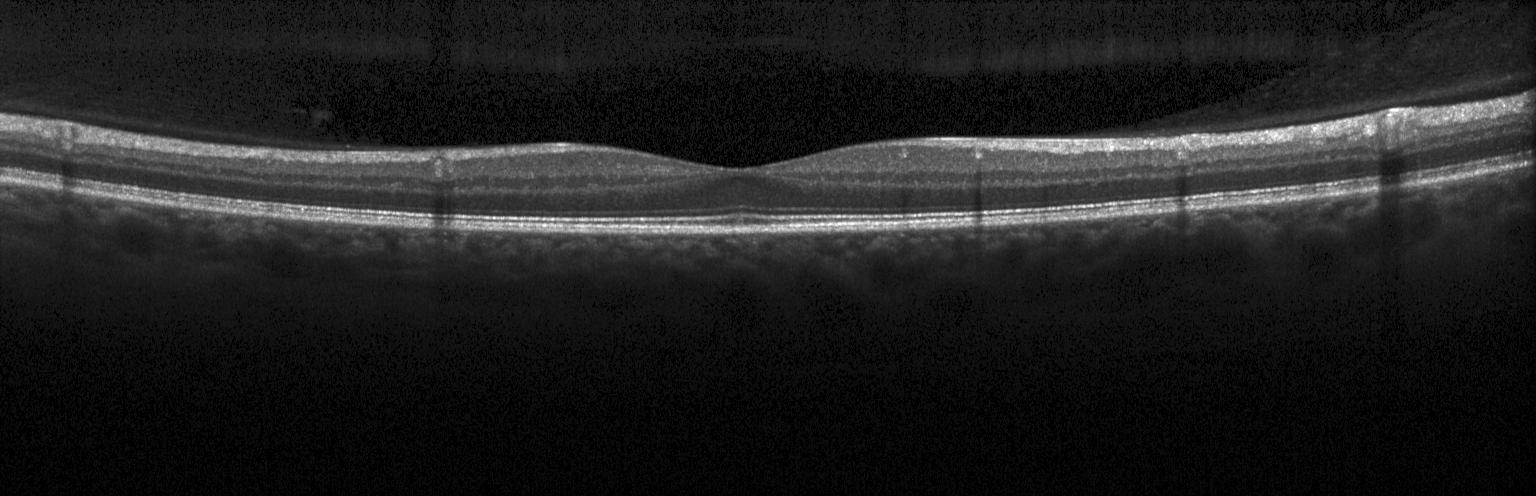
Macular OCT demonstrating no CNV, DME, or drusen.